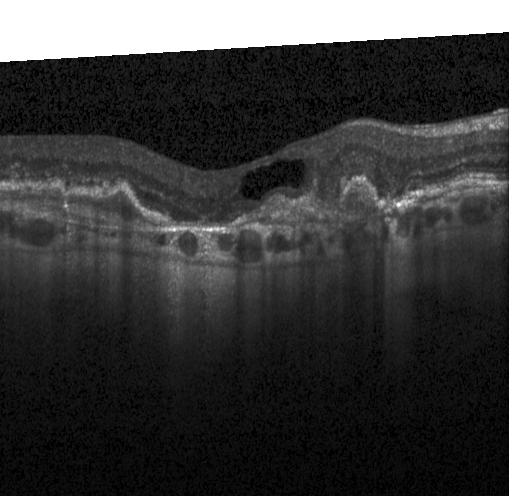
OCT B-scan — This B-scan demonstrates a choroidal neovascular membrane.